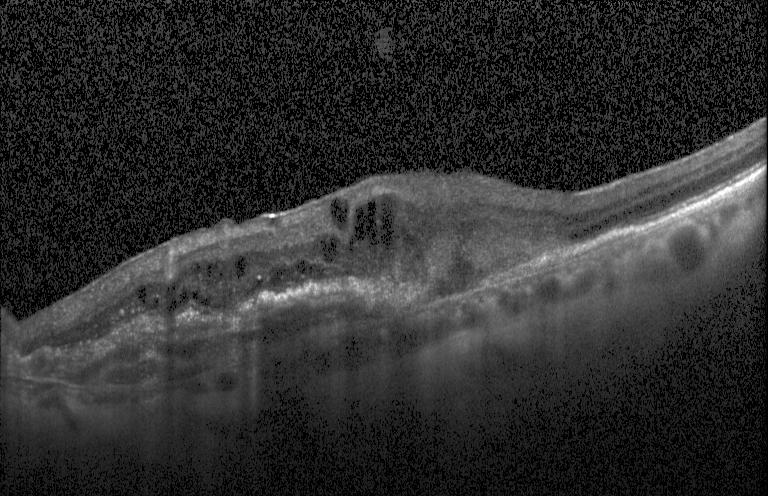
Diagnosis: CNV.